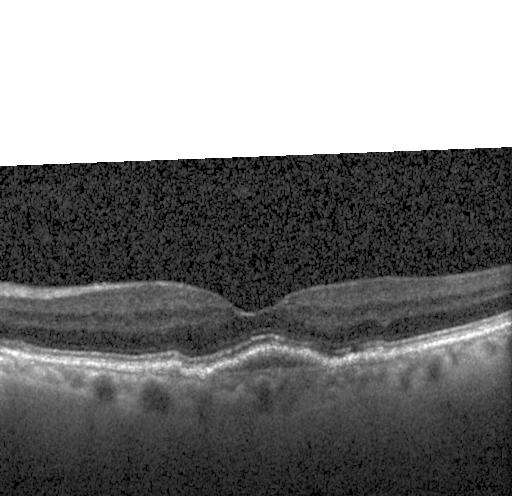

OCT scan showing a choroidal neovascular membrane.